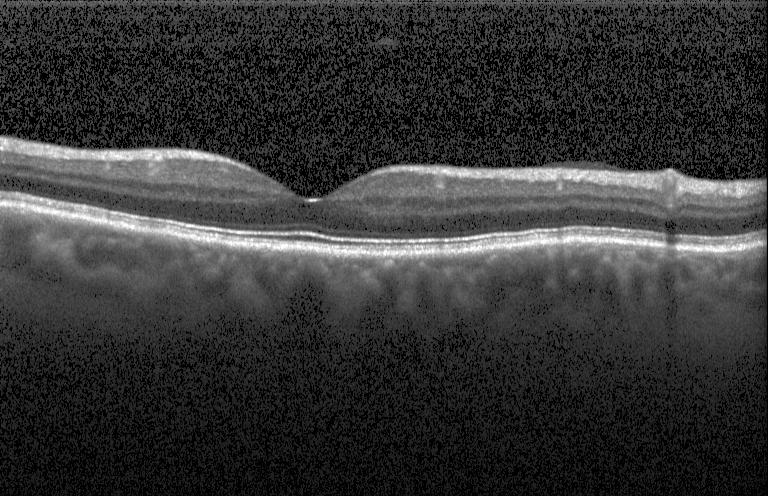

Diagnosis: no evidence of choroidal neovascularization, diabetic macular edema, or drusen.